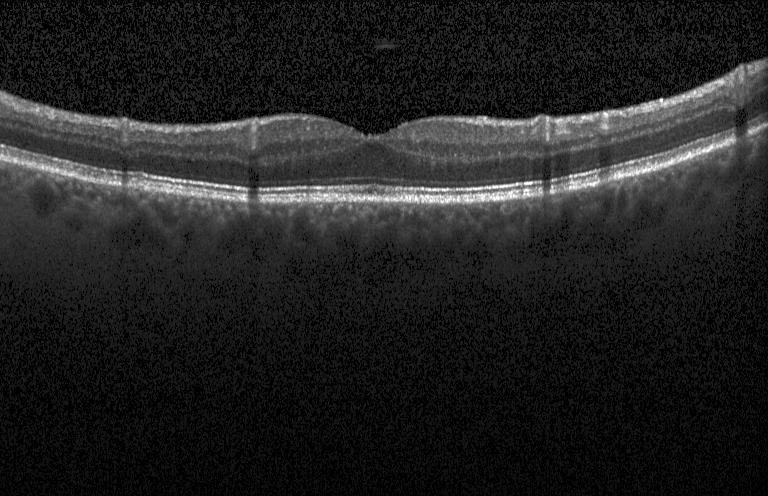 Macular OCT demonstrating no choroidal neovascularization, no diabetic macular edema, and no drusen.